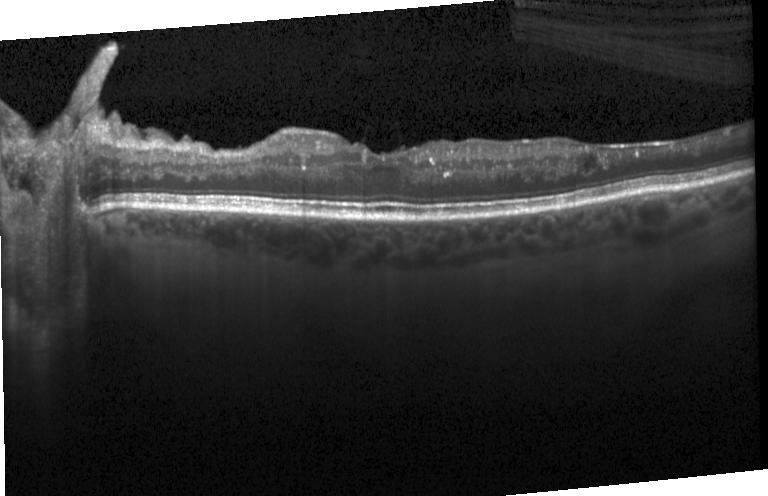 Optical coherence tomography B-scan. Spectral-domain optical coherence tomography. Instrument: Heidelberg Spectralis — Finding: diabetic macular edema.